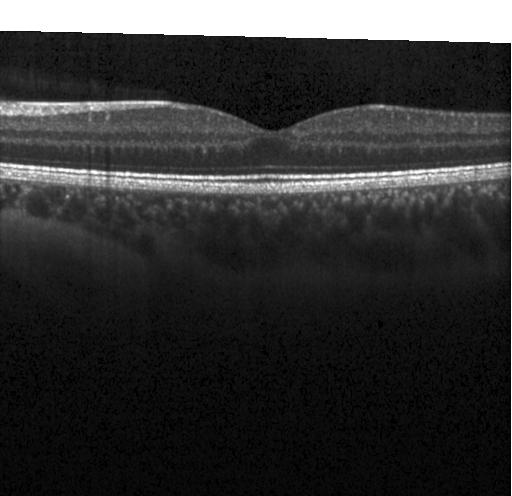 Acquired on a Heidelberg Spectralis, optical coherence tomography B-scan
No evidence of CNV, DME, or drusen.